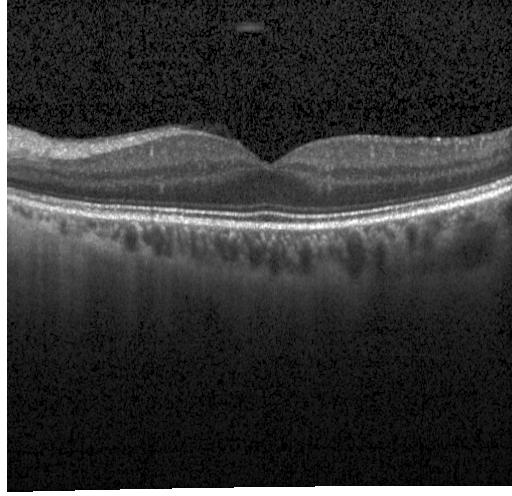

Assessment: no evidence of choroidal neovascularization, diabetic macular edema, or drusen.